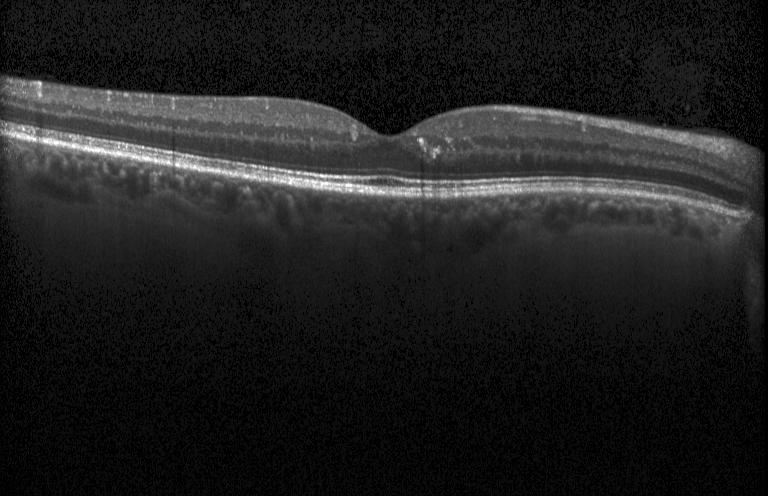

Macular scan · optical coherence tomography scan — Impression: neither choroidal neovascularization, diabetic macular edema, nor drusen.